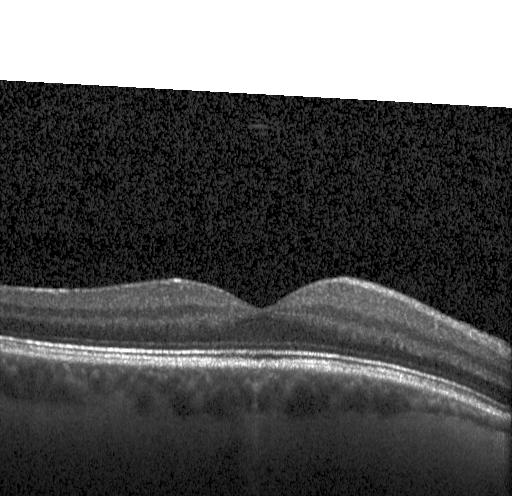 Heidelberg Spectralis, spectral-domain optical coherence tomography, macular scan, optical coherence tomography scan.
Macular OCT: no choroidal neovascularization, no diabetic macular edema, and no drusen.